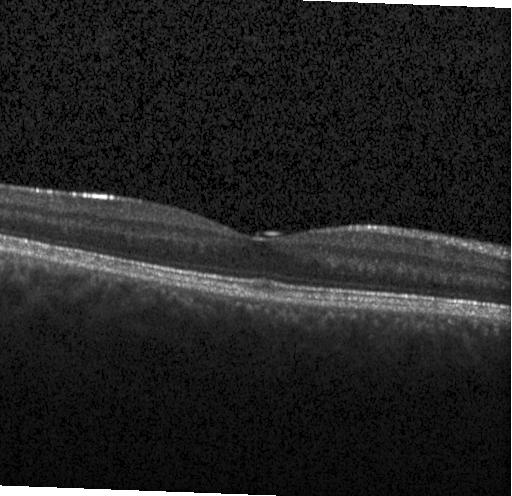
SD-OCT. OCT B-scan. Through the macula. Acquired on a Heidelberg Spectralis
OCT finding: no choroidal neovascularization, diabetic macular edema, or drusen.